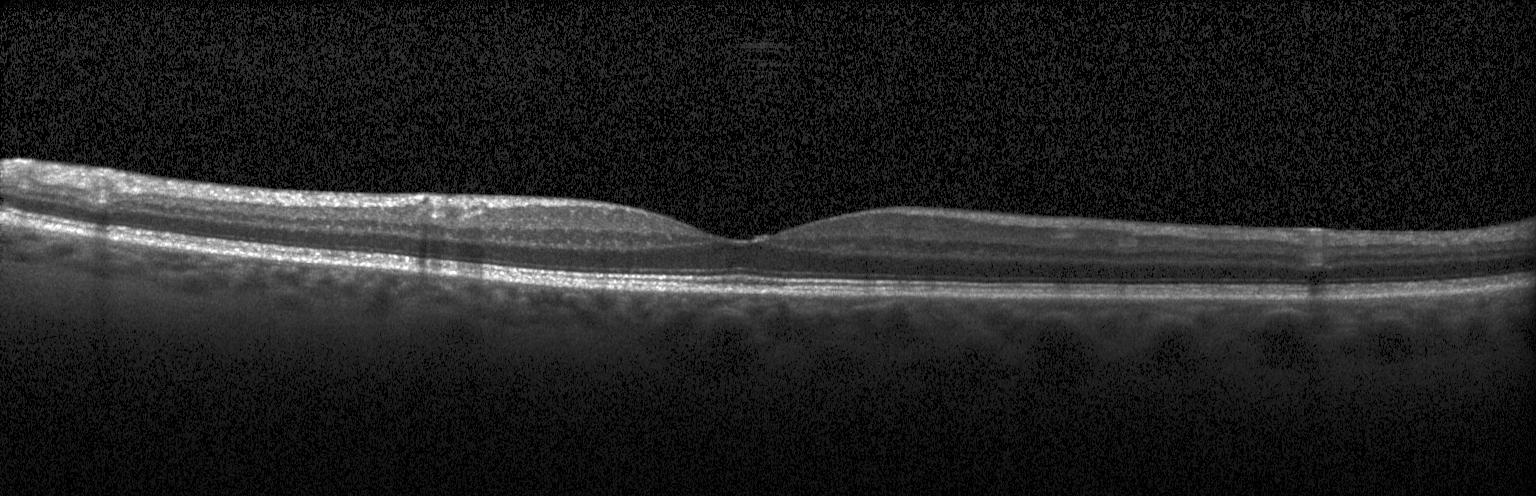
Finding: no evidence of choroidal neovascularization, diabetic macular edema, or drusen.